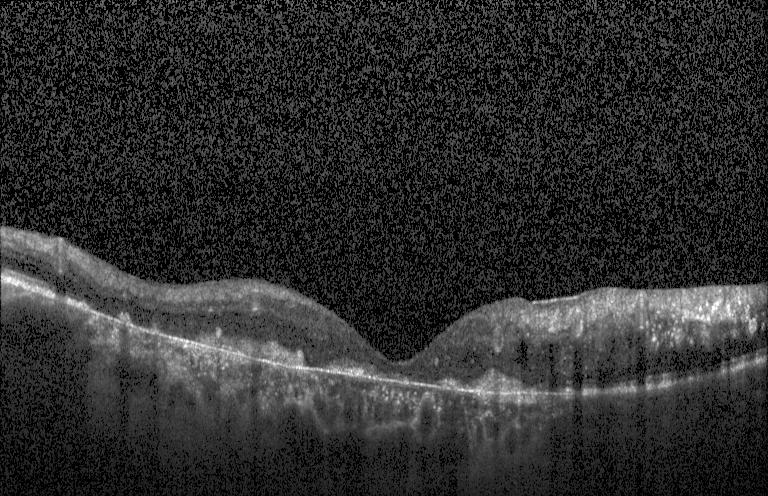

Optical coherence tomography B-scan.
Assessment: CNV.